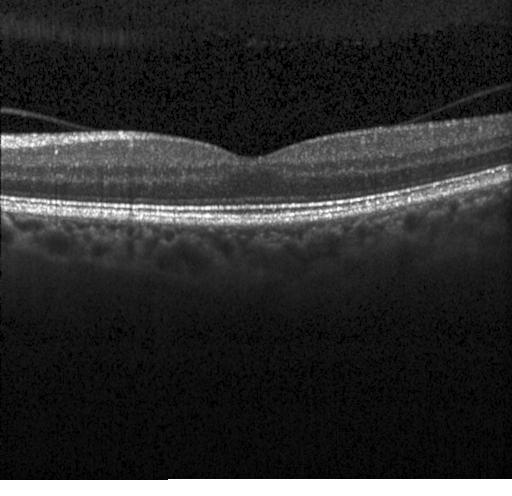
Through the macula; retinal OCT cross-section — This B-scan demonstrates no evidence of CNV, DME, or drusen.